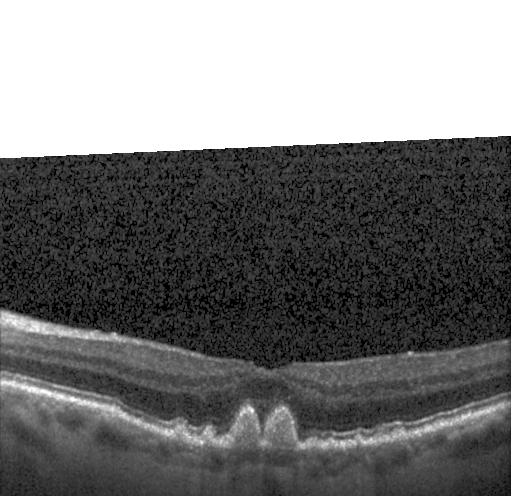
Optical coherence tomography scan. Dx: sub-RPE drusenoid deposits.